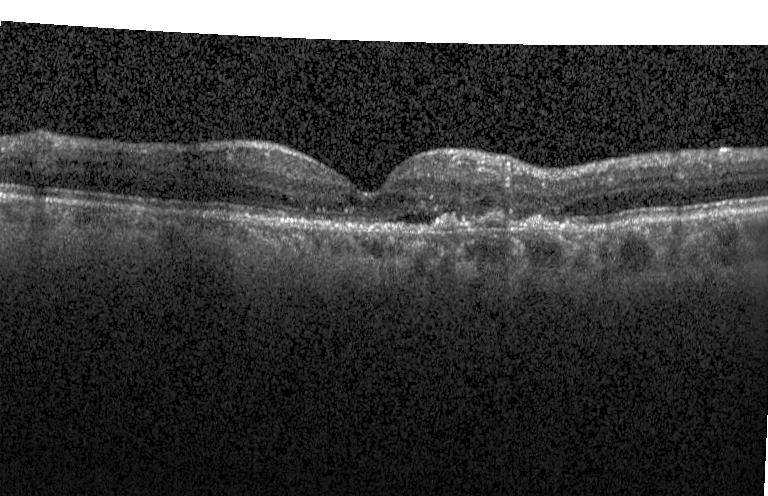

OCT line scan. Spectral-domain optical coherence tomography. Heidelberg Spectralis. Fovea-centered
A choroidal neovascular membrane.